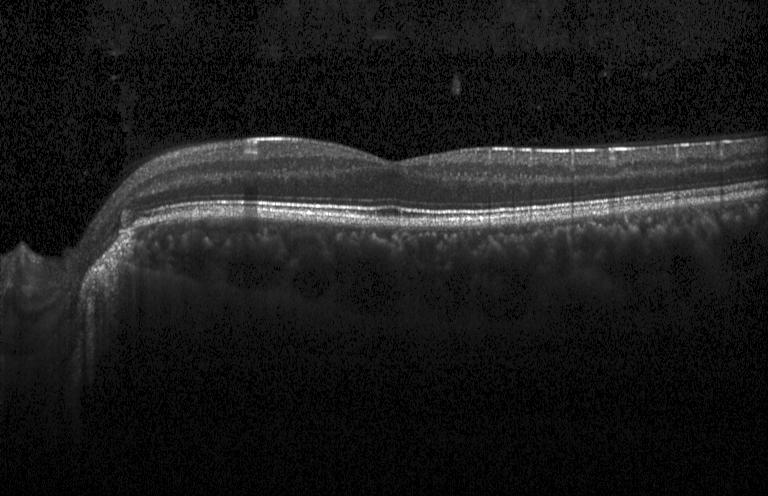

OCT B-scan showing neither choroidal neovascularization, diabetic macular edema, nor drusen.